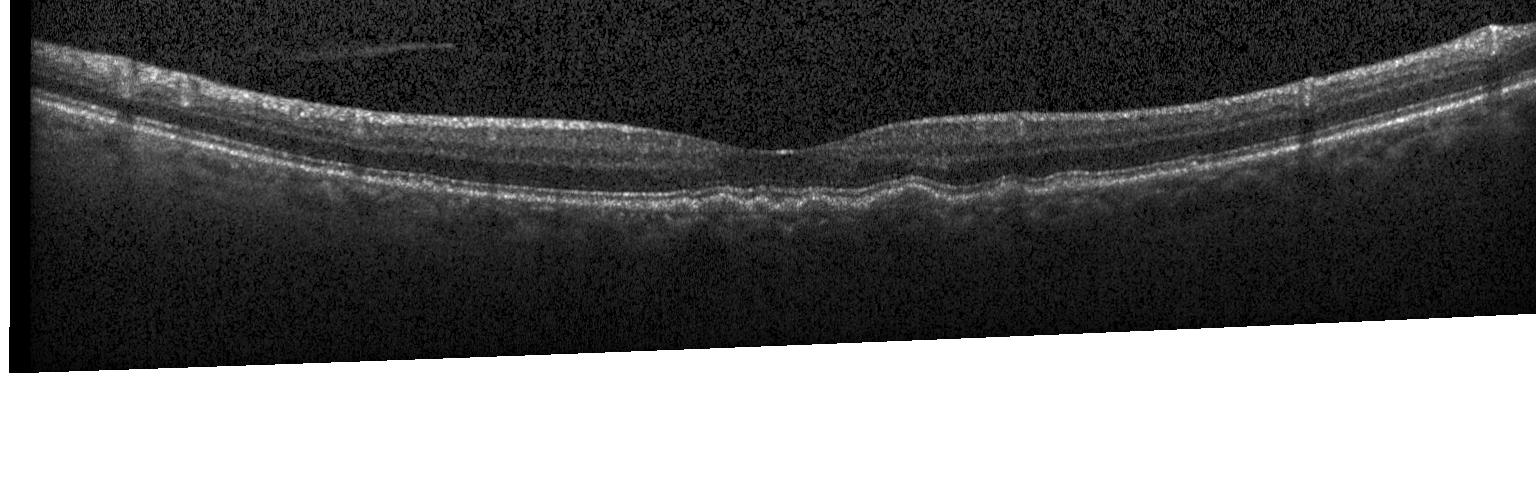 Optical coherence tomography B-scan; centered on the fovea
The scan shows multiple drusen.